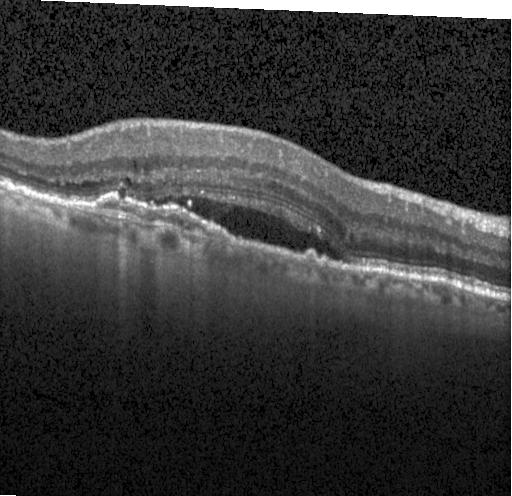 Optical coherence tomography B-scan
Assessment: CNV.